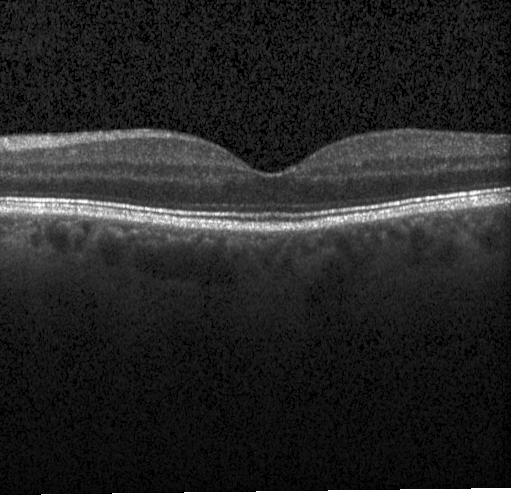
Through the macula; OCT B-scan — Macular OCT: no choroidal neovascularization, diabetic macular edema, or drusen.